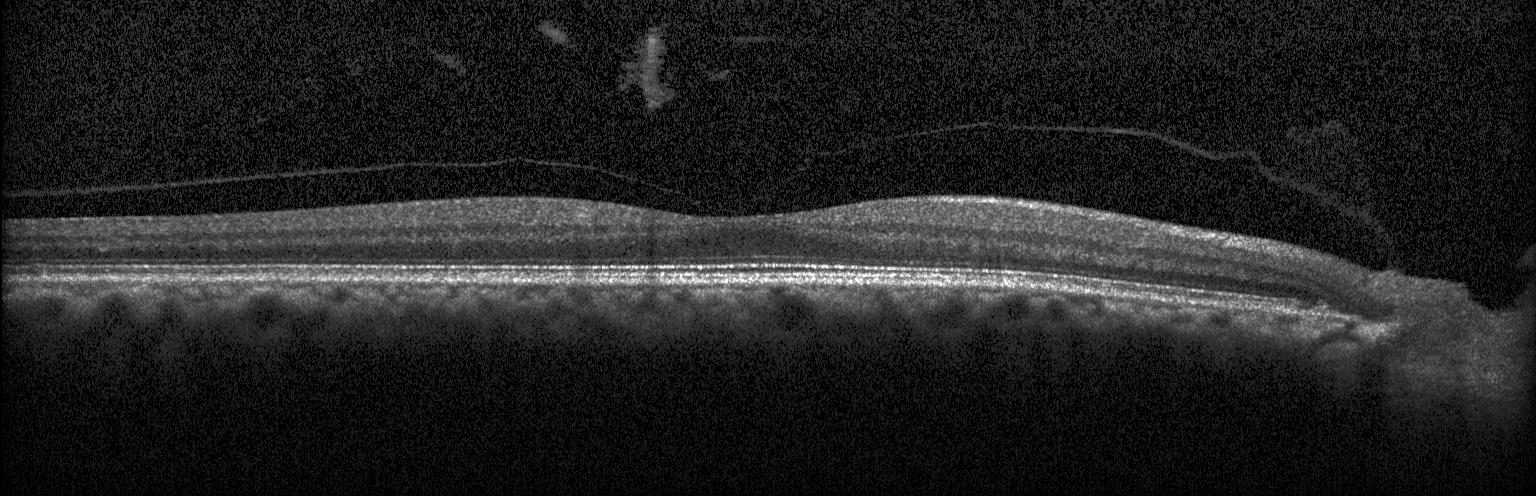 OCT line scan · spectral-domain OCT · acquired on a Heidelberg Spectralis. Macular OCT: no choroidal neovascularization, no diabetic macular edema, and no drusen.